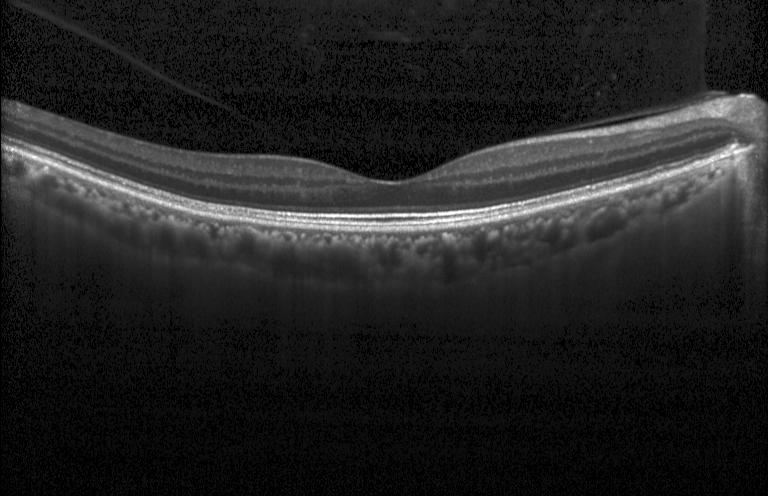

OCT scan showing no choroidal neovascularization, diabetic macular edema, or drusen.